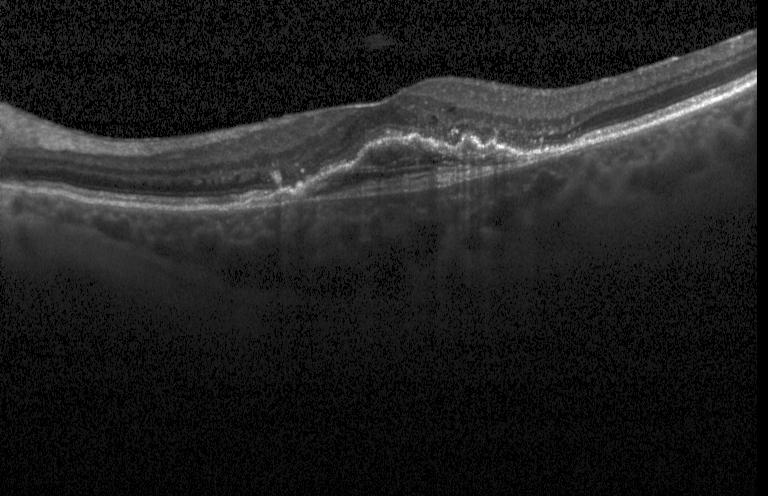 Diagnosis: a choroidal neovascular membrane.